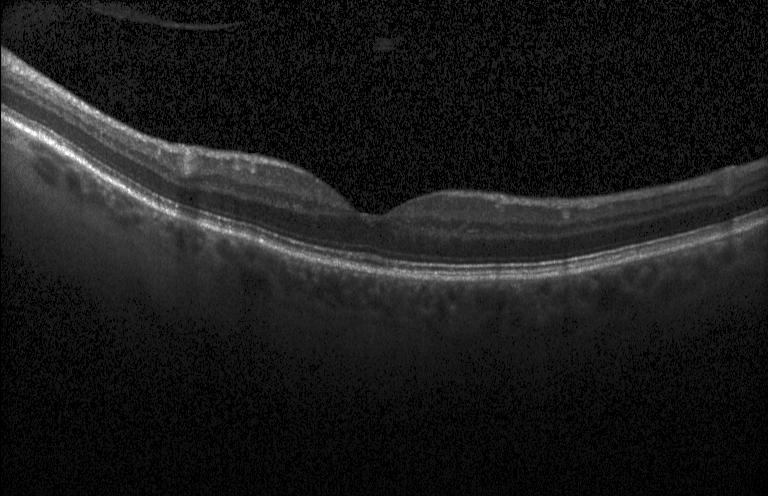
Through the macula, spectral-domain optical coherence tomography, optical coherence tomography B-scan.
Assessment: no CNV, no DME, and no drusen.